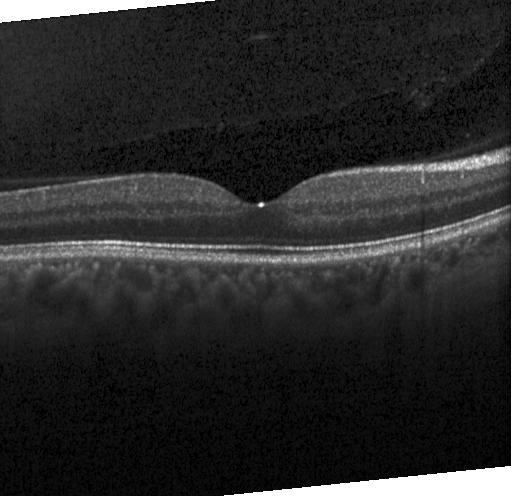
OCT line scan. Assessment: no evidence of choroidal neovascularization, diabetic macular edema, or drusen.